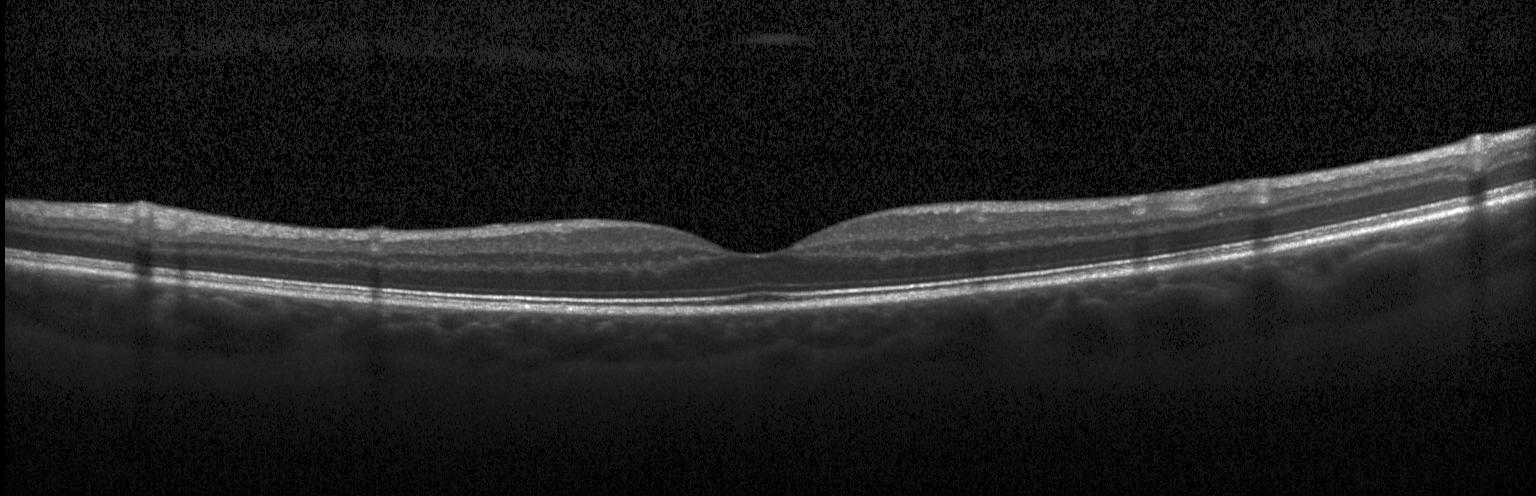

Retinal OCT B-scan. Finding: no evidence of choroidal neovascularization, diabetic macular edema, or drusen.